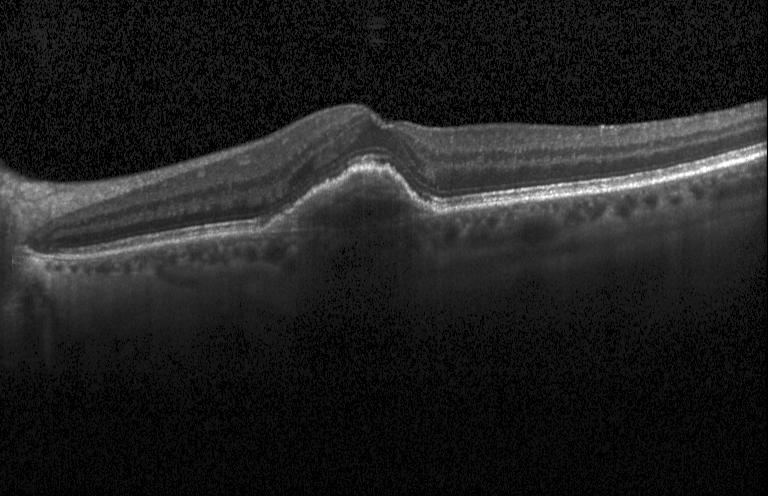 Dx: CNV.